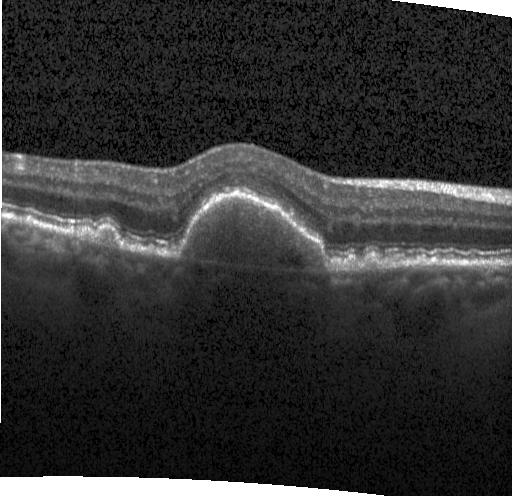

Finding: CNV.